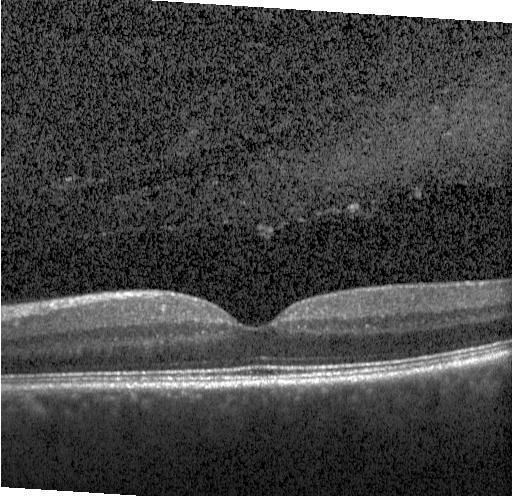
Retinal OCT cross-section showing no choroidal neovascularization, diabetic macular edema, or drusen.